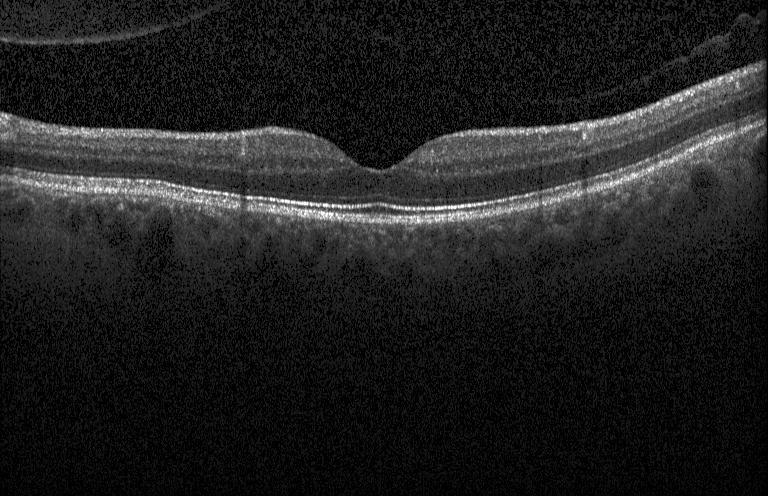
OCT line scan · fovea-centered · SD-OCT · Heidelberg Spectralis OCT system. Finding: no choroidal neovascularization, no diabetic macular edema, and no drusen.